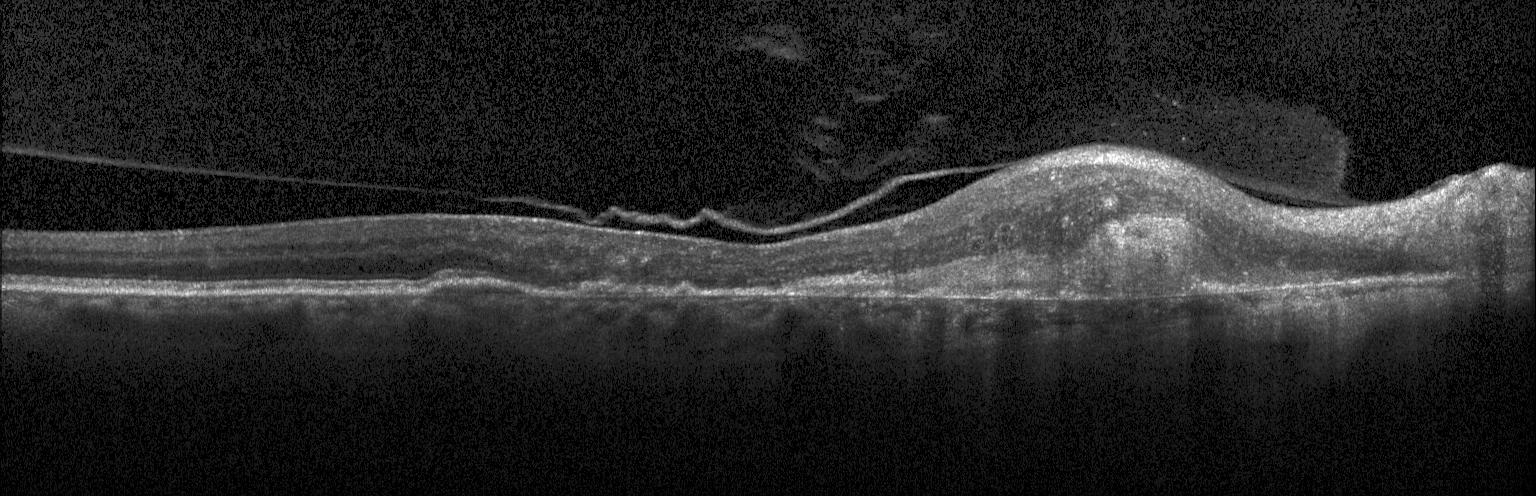 Acquired on a Heidelberg Spectralis; macular scan; retinal OCT B-scan
Impression: a choroidal neovascular membrane.